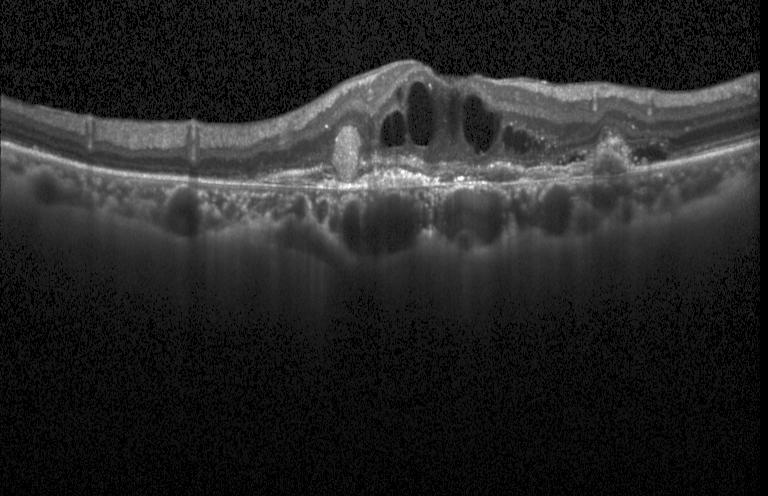

Optical coherence tomography B-scan — Finding: a choroidal neovascular membrane.